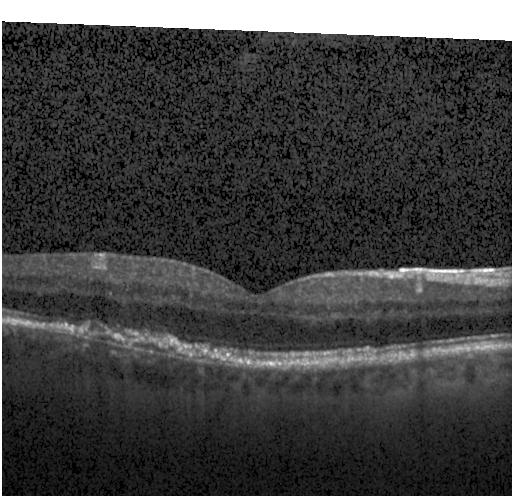

Retinal OCT cross-section showing multiple drusen.